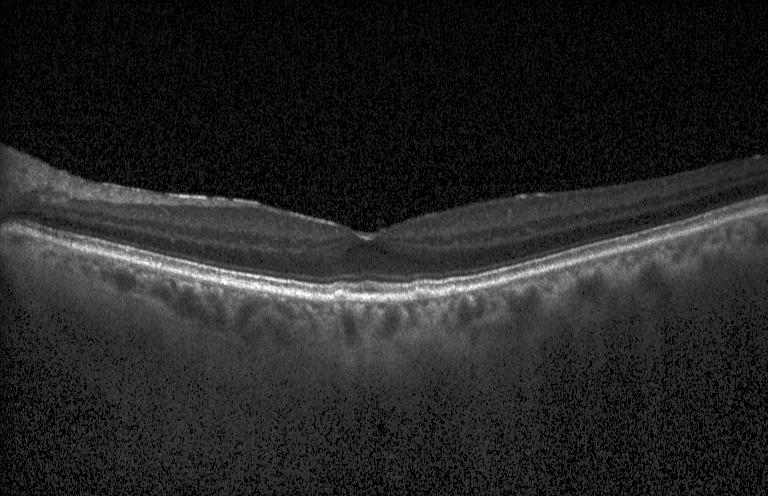 Retinal OCT cross-section showing multiple drusen.